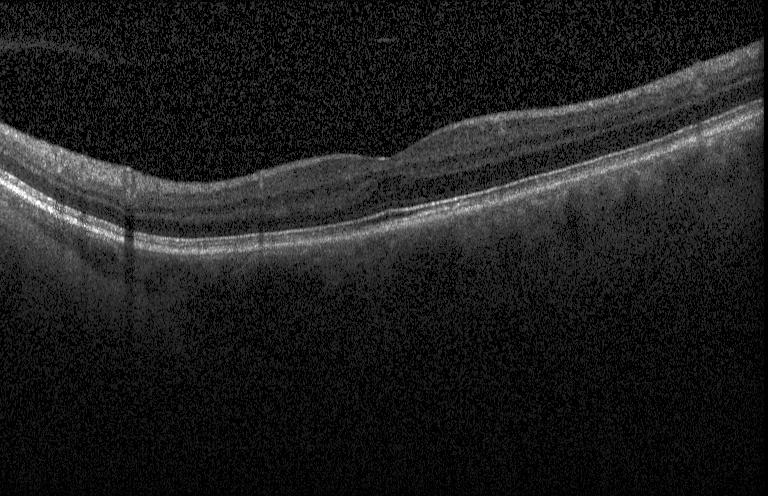 Spectral-domain OCT. Instrument: Heidelberg Spectralis. Retinal OCT cross-section. Through the macula
This B-scan demonstrates no CNV, no DME, and no drusen.